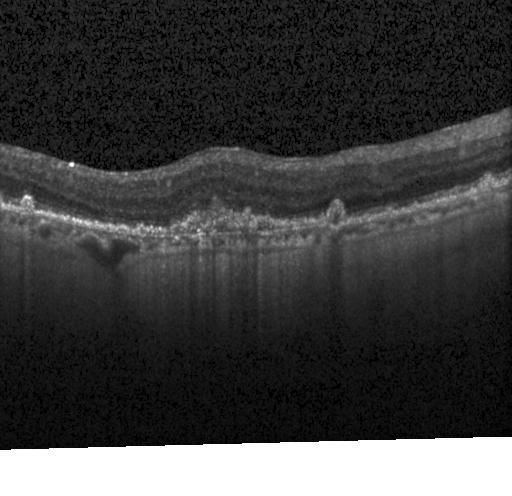
Diagnosis: a choroidal neovascular membrane.